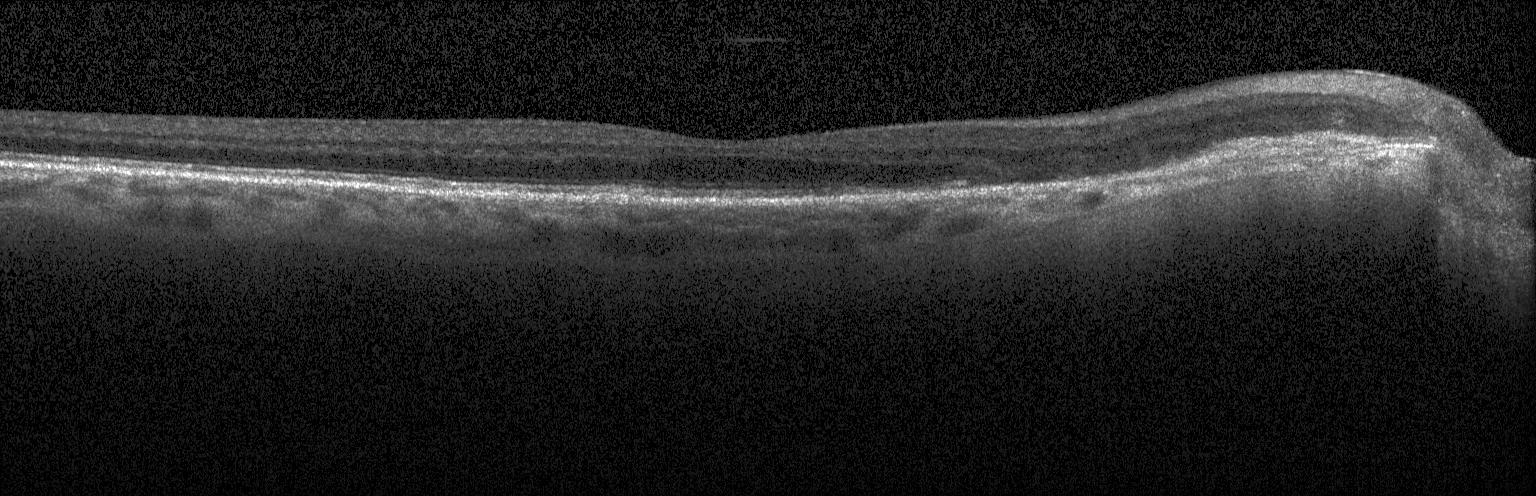
Spectral-domain OCT B-scan: choroidal neovascularization (CNV).